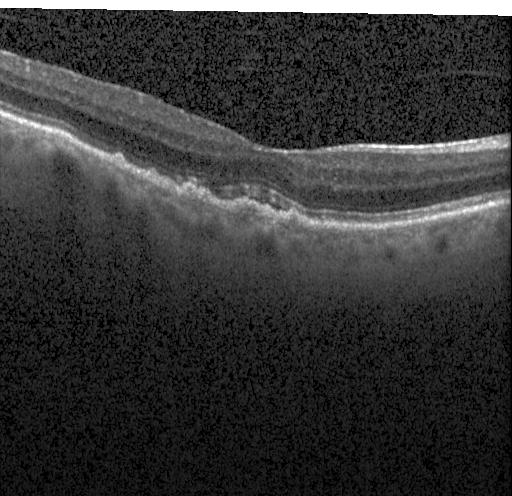
SD-OCT, optical coherence tomography scan. Macular OCT: choroidal neovascularization.